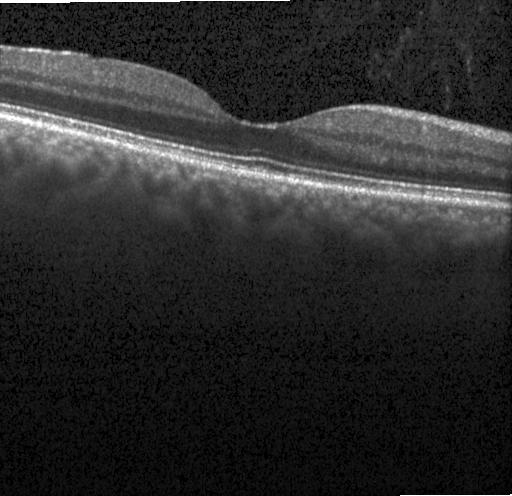

Retinal OCT B-scan.
The scan shows no CNV, DME, or drusen.